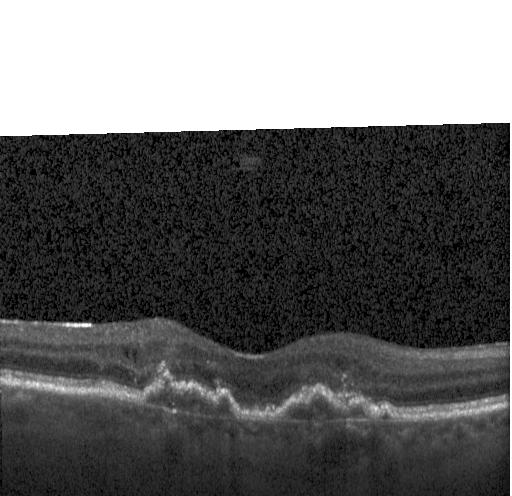 Finding: choroidal neovascularization.